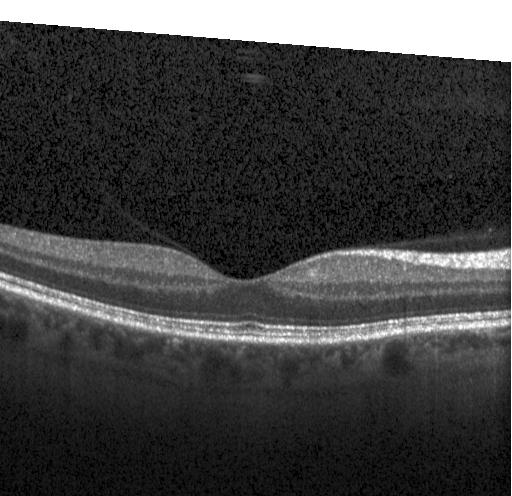

Centered on the fovea · optical coherence tomography B-scan — Diagnosis: neither choroidal neovascularization, diabetic macular edema, nor drusen.